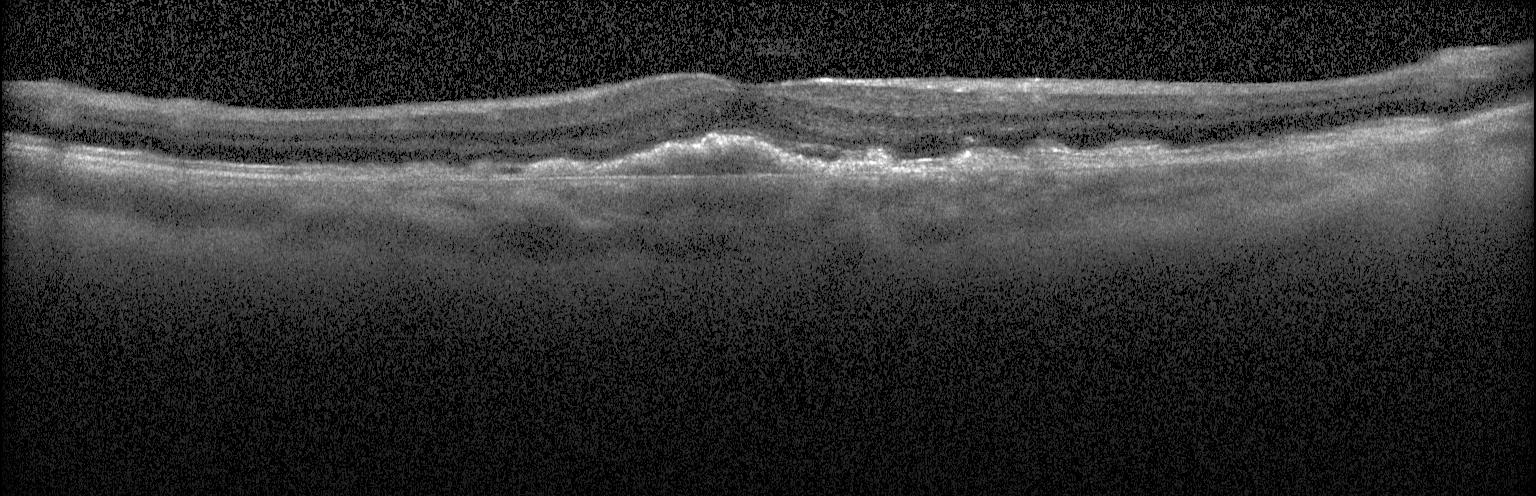

Finding: a choroidal neovascular membrane.